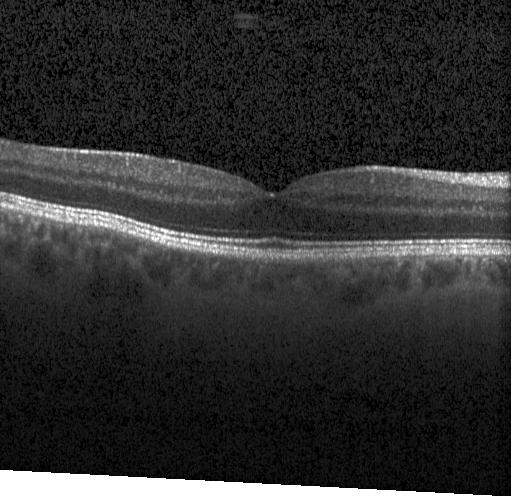

Dx: no evidence of choroidal neovascularization, diabetic macular edema, or drusen.